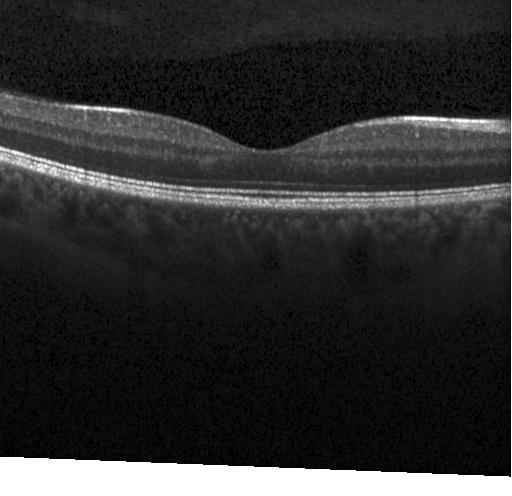 This B-scan demonstrates no choroidal neovascularization, diabetic macular edema, or drusen.